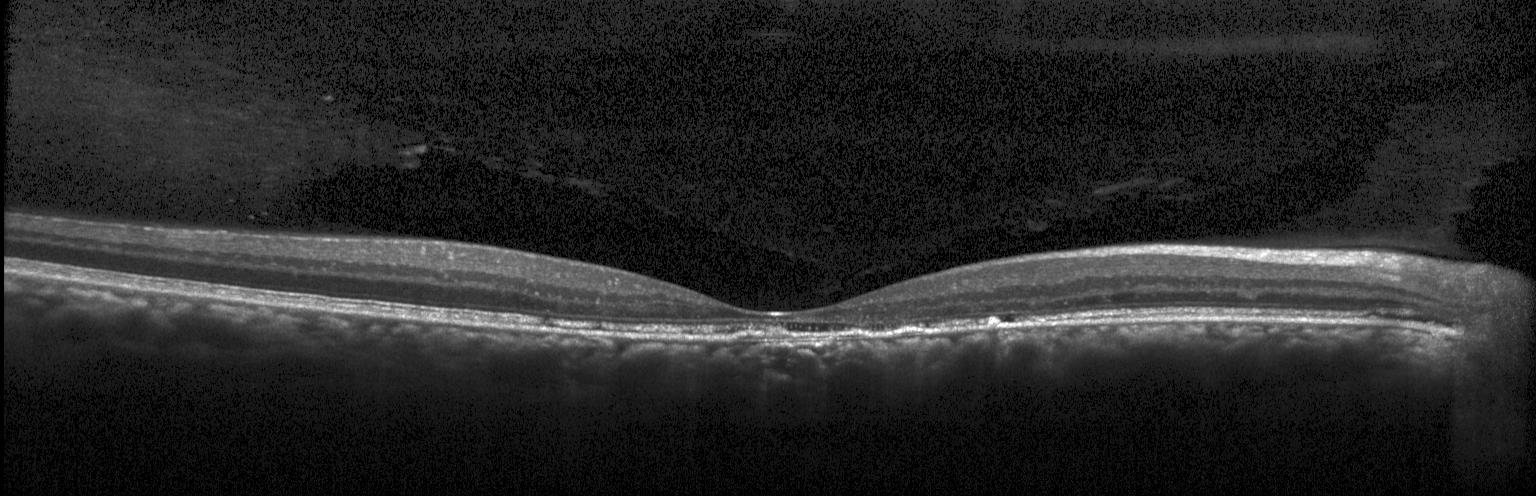

Spectral-domain OCT, instrument: Heidelberg Spectralis, horizontal scan through the fovea, OCT B-scan. Finding: CNV.